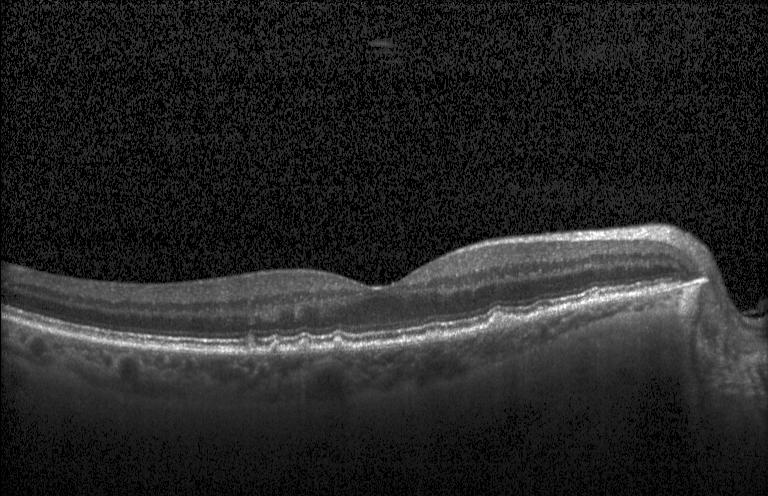

OCT scan showing drusen.